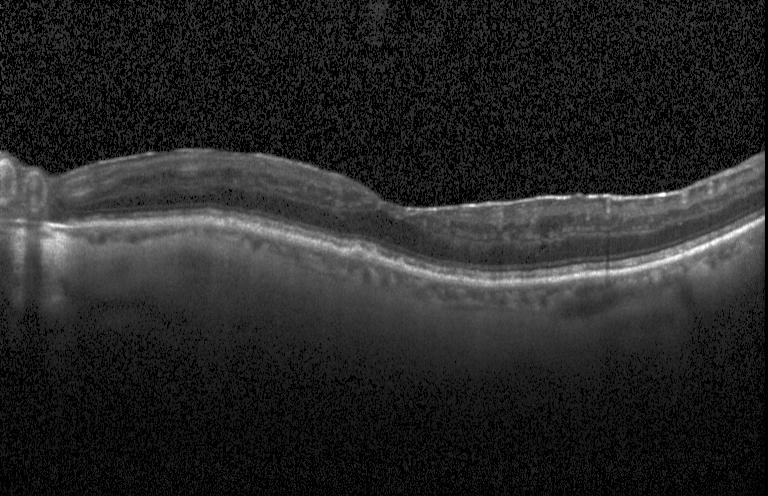 Optical coherence tomography B-scan. Heidelberg Spectralis OCT system. SD-OCT. Centered on the fovea
Macular OCT: sub-RPE drusenoid deposits.